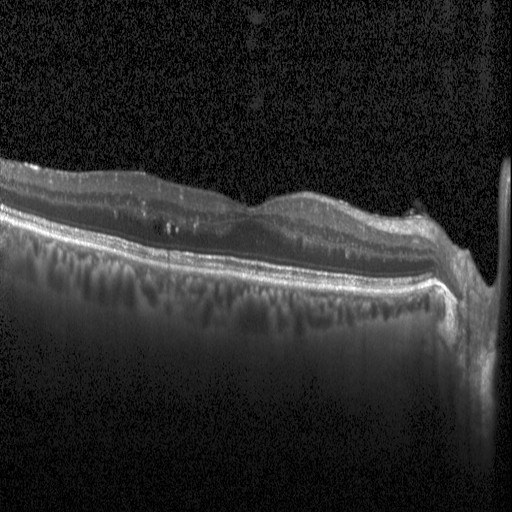 Impression: diabetic macular edema.